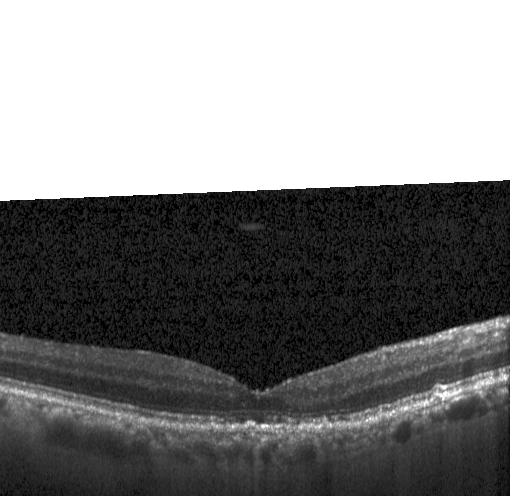

OCT scan showing sub-RPE drusenoid deposits.